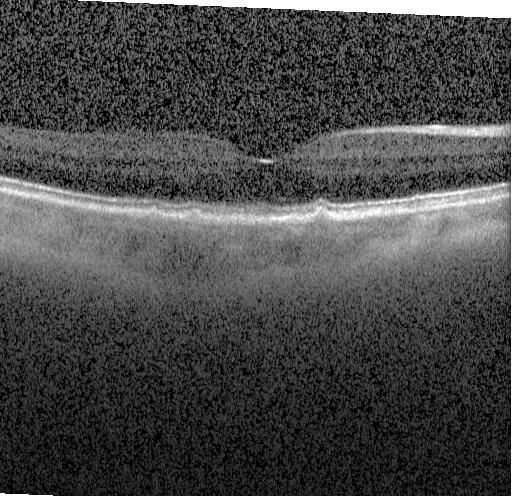

Retinal OCT cross-section
Impression: drusen.